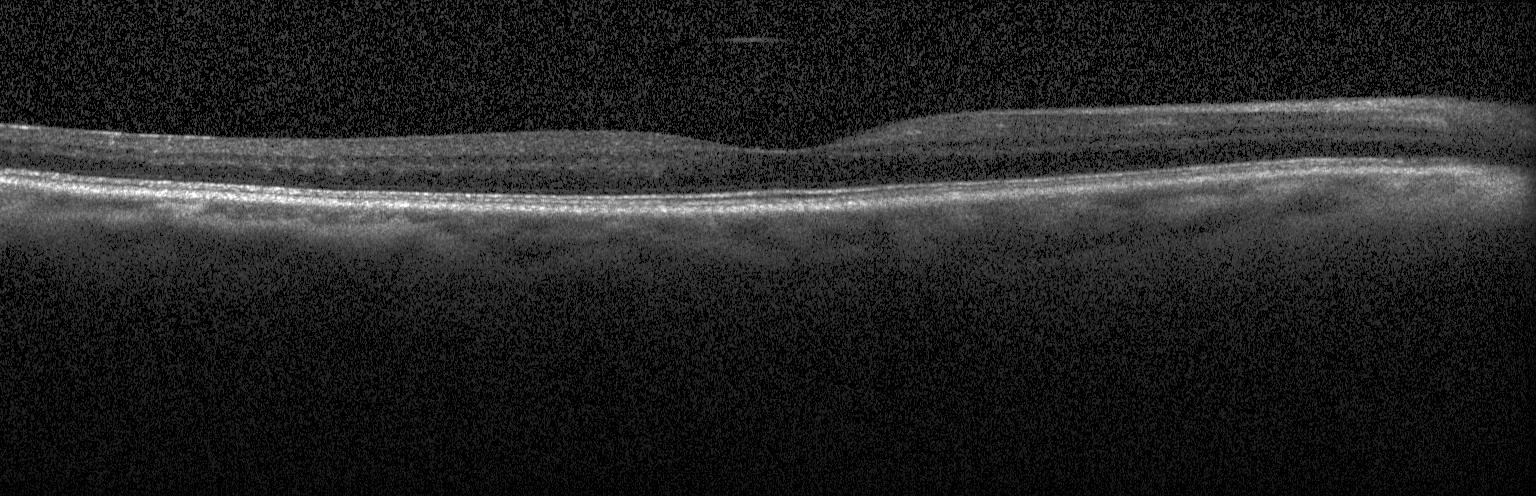 Optical coherence tomography B-scan.
Impression: neither choroidal neovascularization, diabetic macular edema, nor drusen.